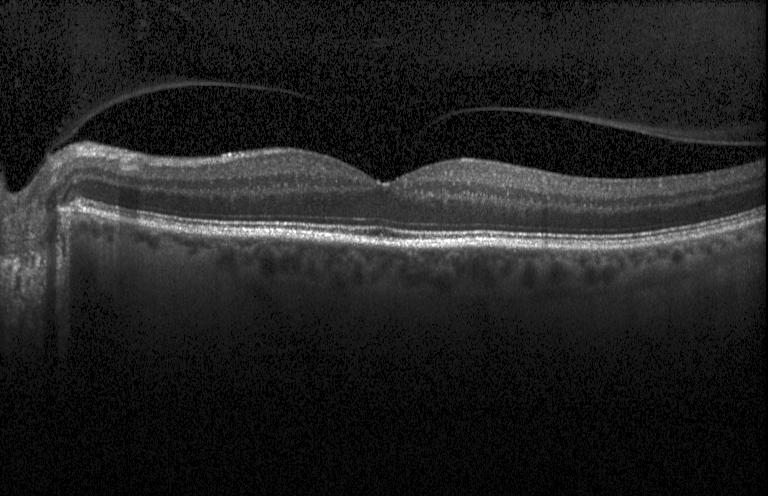
Retinal OCT B-scan · spectral-domain OCT — Macular OCT: no evidence of choroidal neovascularization, diabetic macular edema, or drusen.